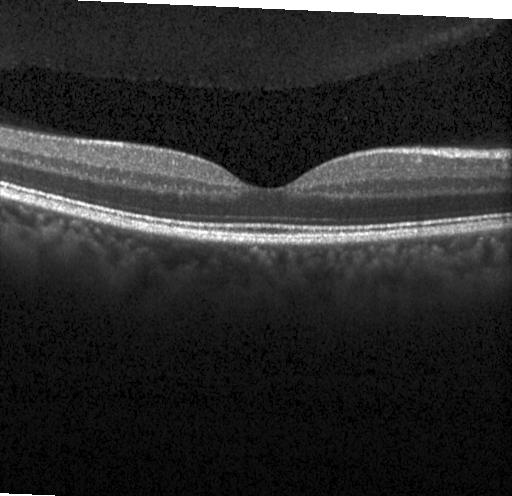

OCT B-scan; through the macula. Dx: neither choroidal neovascularization, diabetic macular edema, nor drusen.